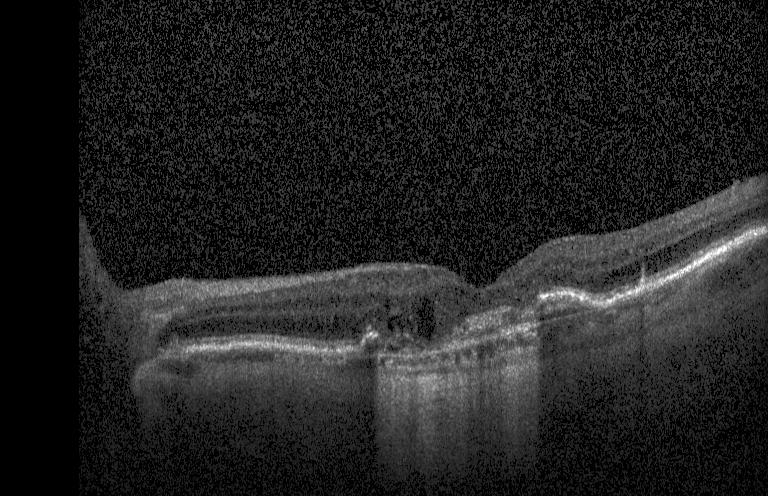

Diagnosis: a choroidal neovascular membrane.